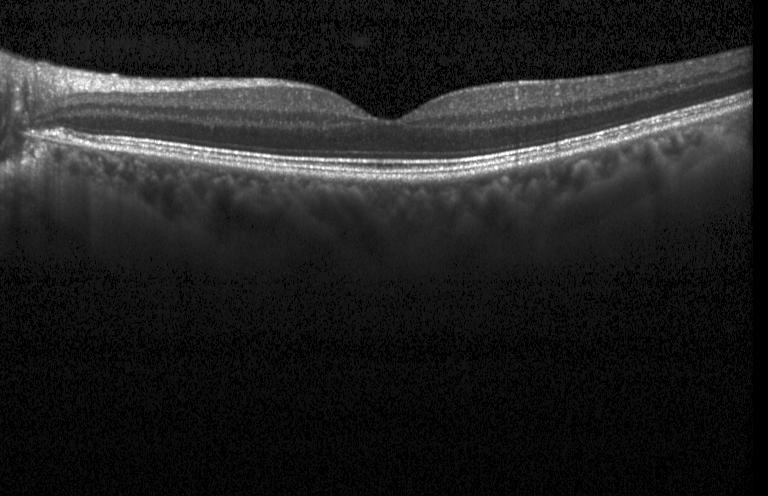
Optical coherence tomography scan. Spectral-domain optical coherence tomography. Horizontal scan through the fovea. Heidelberg Spectralis OCT system.
Impression: no evidence of choroidal neovascularization, diabetic macular edema, or drusen.